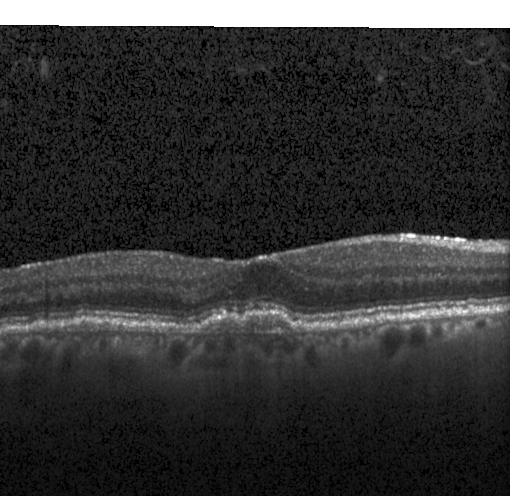 The scan shows a choroidal neovascular membrane.